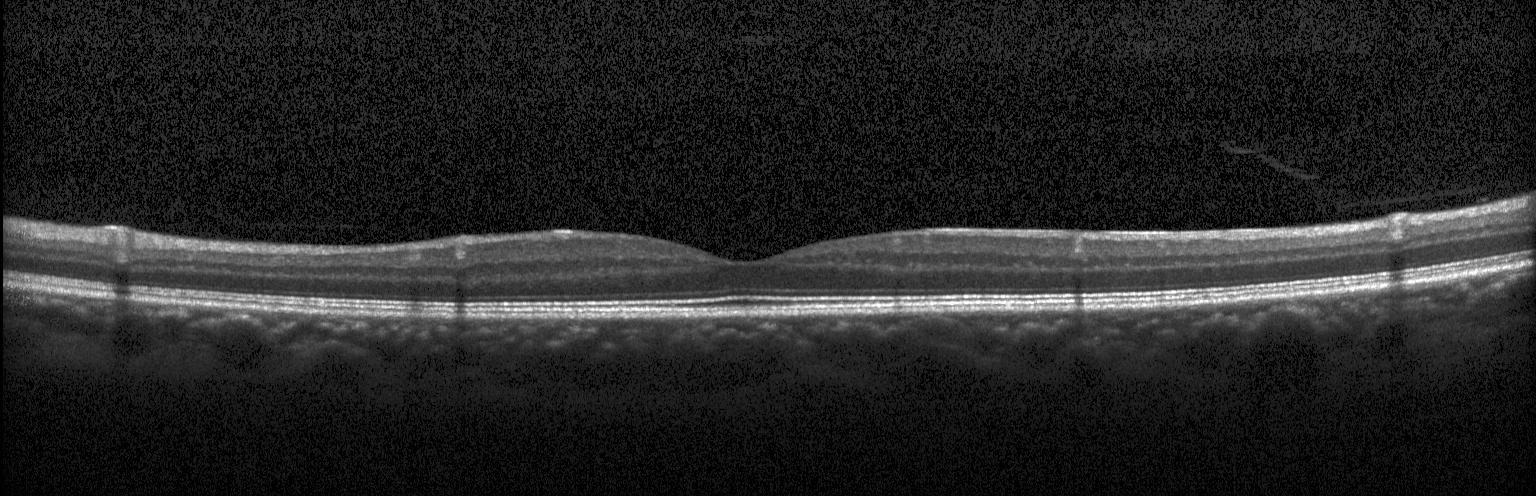 OCT scan showing no choroidal neovascularization, diabetic macular edema, or drusen.